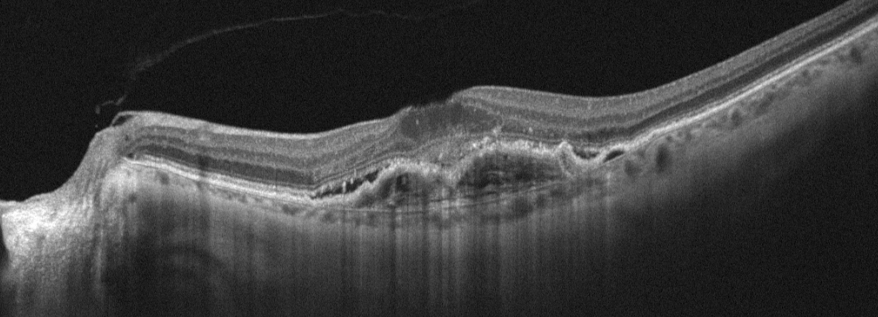

Fovea-centered · Optovue Avanti RTVue XR · optical coherence tomography scan.
Assessment: age-related macular degeneration.